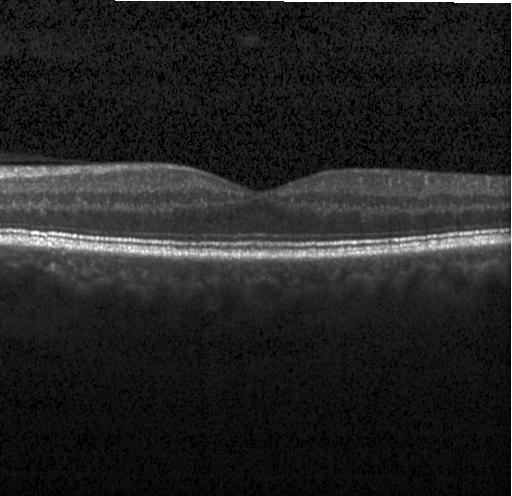

OCT B-scan
The scan shows no choroidal neovascularization, no diabetic macular edema, and no drusen.